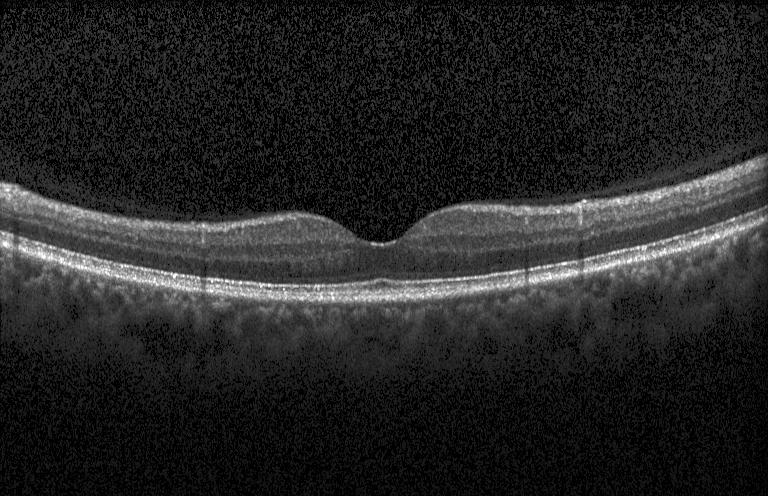 Diagnosis: no CNV, DME, or drusen.